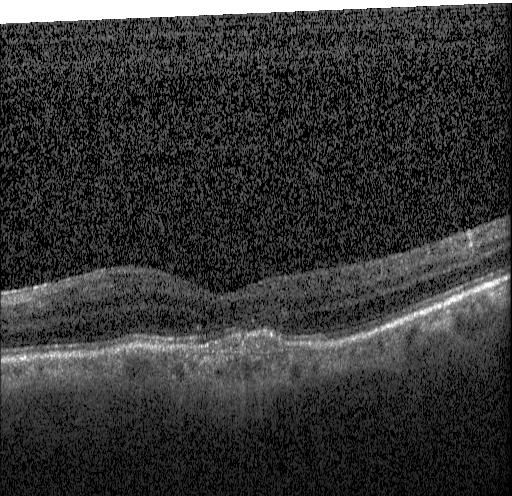 Spectral-domain OCT B-scan: CNV.